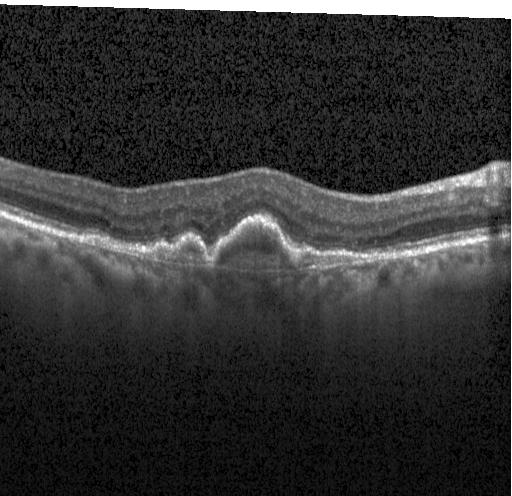
Through the macula; retinal OCT cross-section; SD-OCT.
Diagnosis: a choroidal neovascular membrane.